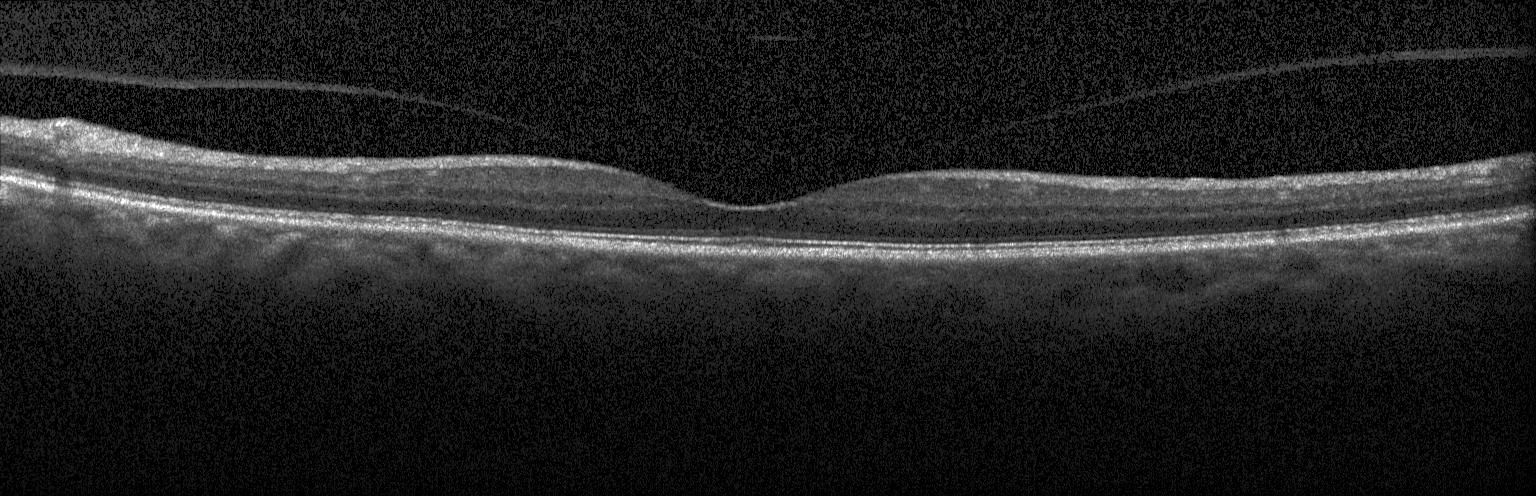
Optical coherence tomography B-scan
Diagnosis: no evidence of CNV, DME, or drusen.